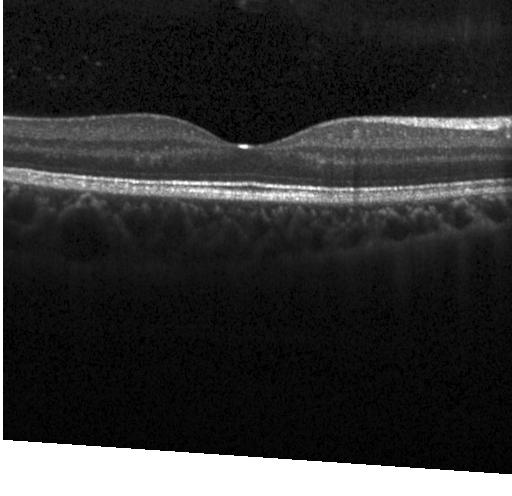 Diagnosis: neither CNV, DME, nor drusen.